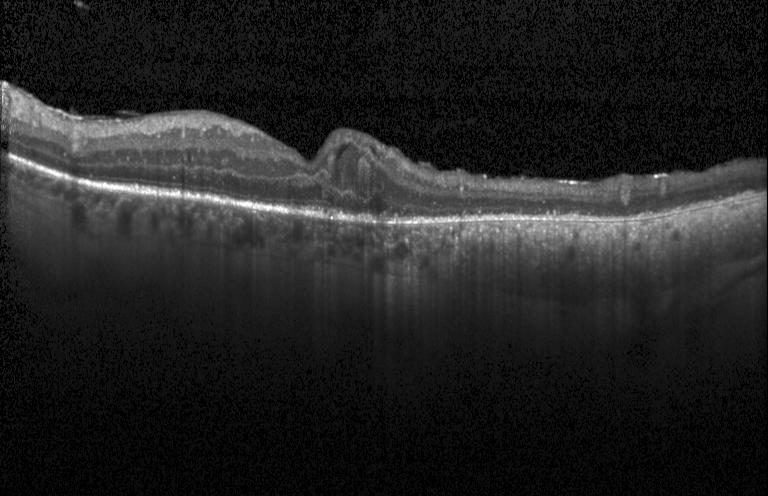

OCT line scan — Diagnosis: diabetic macular edema (DME).